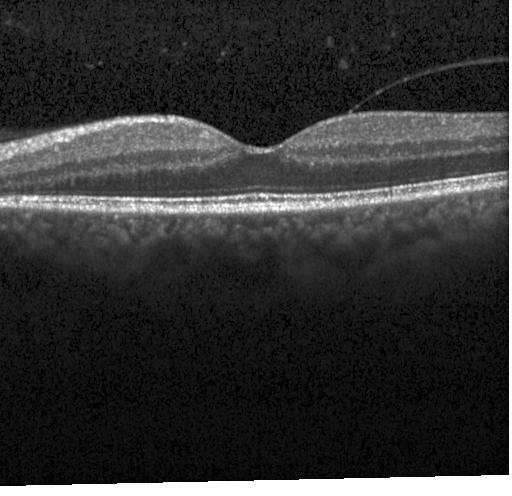

Spectral-domain OCT, retinal OCT cross-section. The scan shows no evidence of choroidal neovascularization, diabetic macular edema, or drusen.